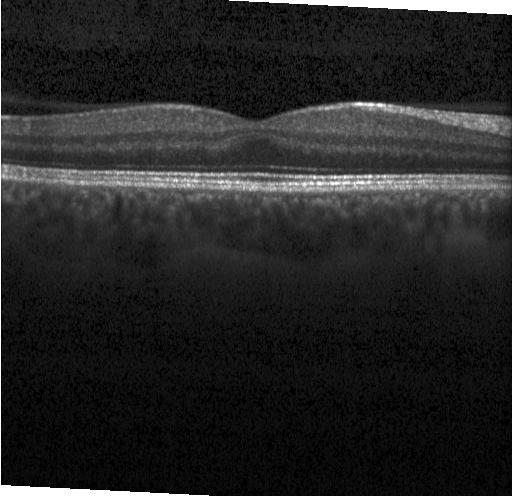 Spectral-domain optical coherence tomography, optical coherence tomography B-scan.
No choroidal neovascularization, no diabetic macular edema, and no drusen.